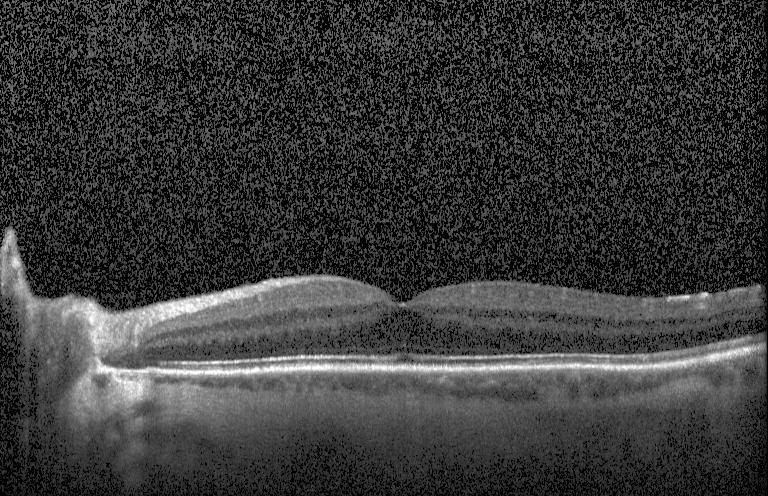 Diagnosis: no choroidal neovascularization, diabetic macular edema, or drusen.